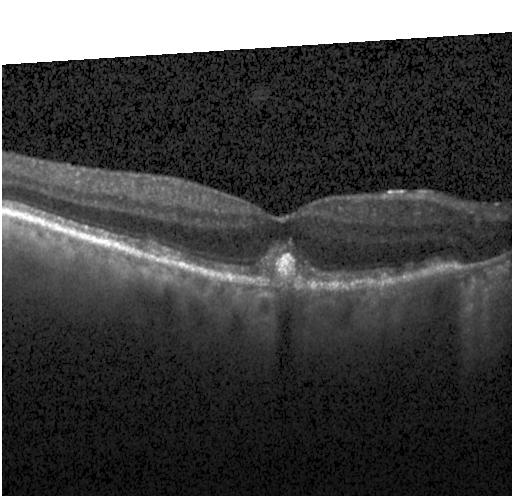

Macular OCT: choroidal neovascularization.